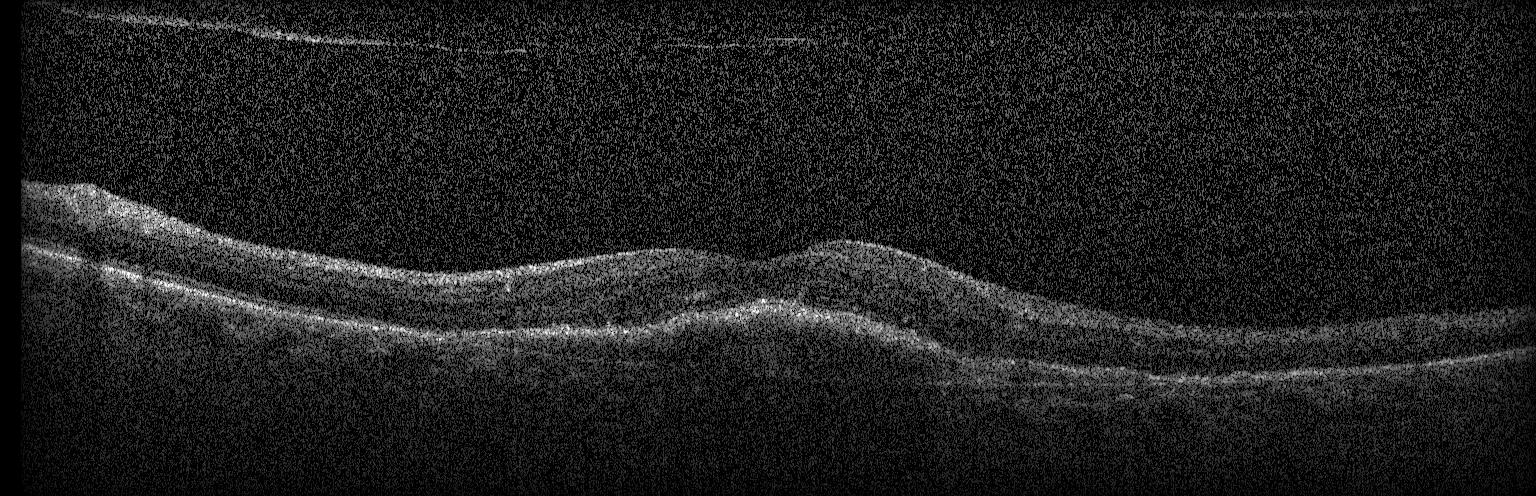

Retinal OCT B-scan, spectral-domain optical coherence tomography, Heidelberg Spectralis
Finding: CNV.